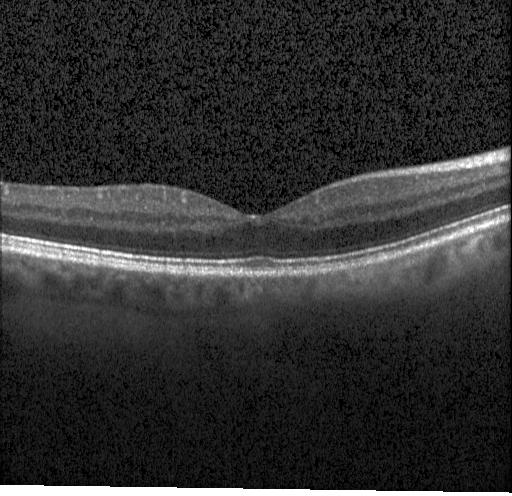 Retinal OCT cross-section.
OCT finding: no choroidal neovascularization, diabetic macular edema, or drusen.